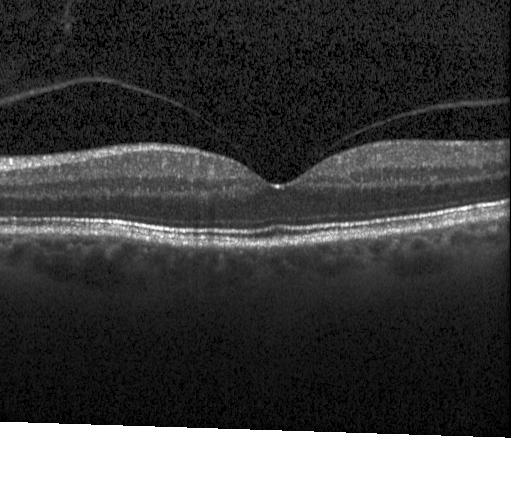 Instrument: Heidelberg Spectralis. SD-OCT. Optical coherence tomography B-scan. Macular scan — OCT finding: neither choroidal neovascularization, diabetic macular edema, nor drusen.